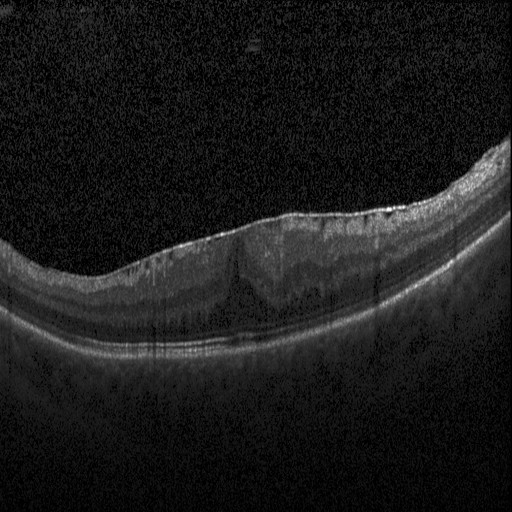
Retinal OCT cross-section, Heidelberg Spectralis, spectral-domain optical coherence tomography.
Macular OCT: diabetic macular edema (DME).